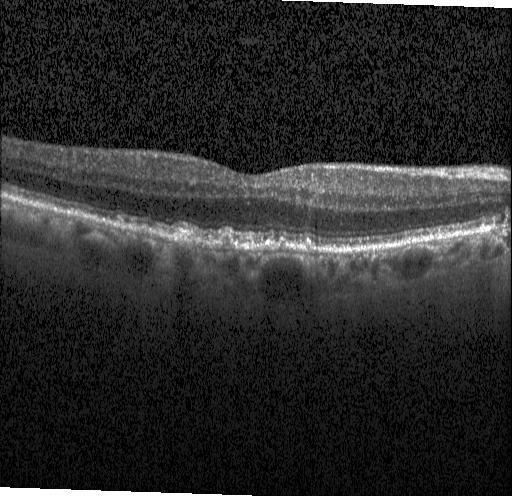 Optical coherence tomography B-scan, centered on the fovea, SD-OCT
Macular OCT: multiple drusen.